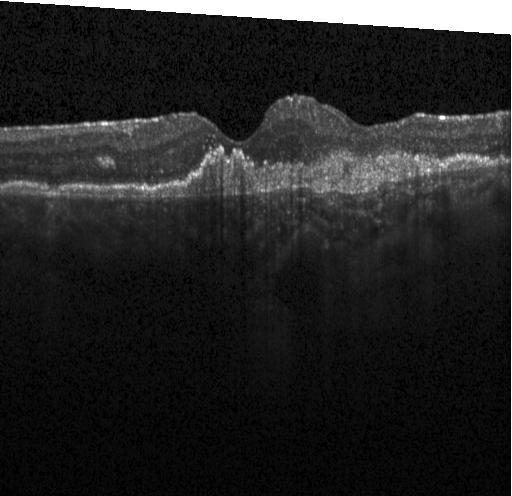
Optical coherence tomography B-scan. Fovea-centered — Finding: choroidal neovascularization (CNV).